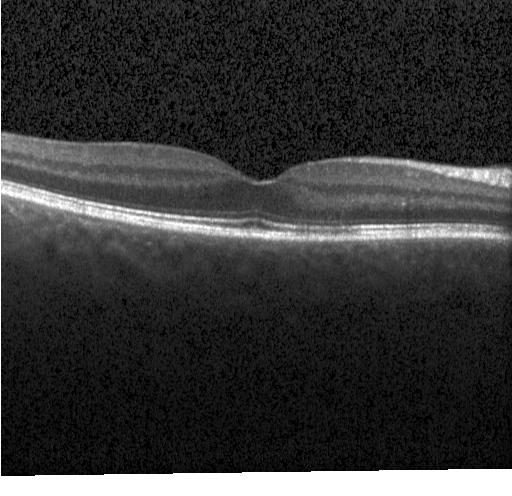 Spectral-domain optical coherence tomography · fovea-centered · optical coherence tomography scan
The scan shows no choroidal neovascularization, no diabetic macular edema, and no drusen.